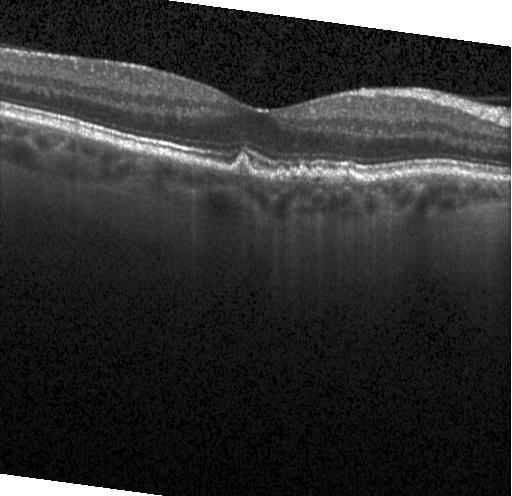
Macular OCT: multiple drusen.